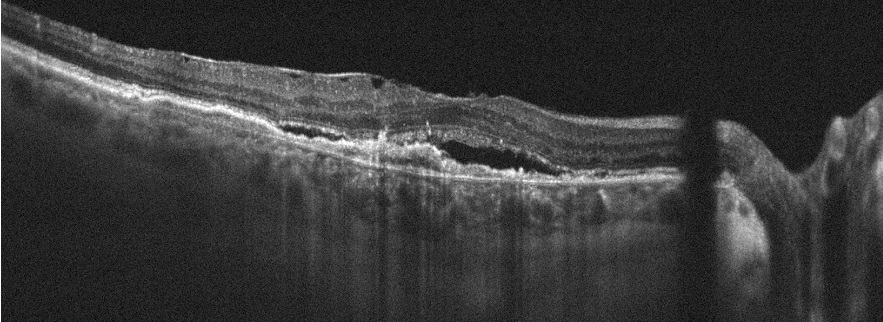
Assessment: AMD.